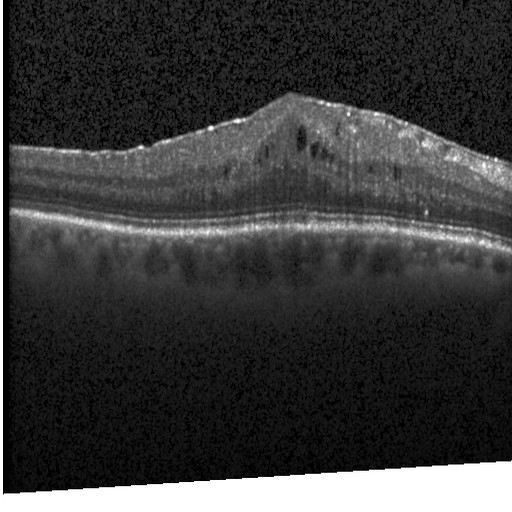
Diagnosis: DME.